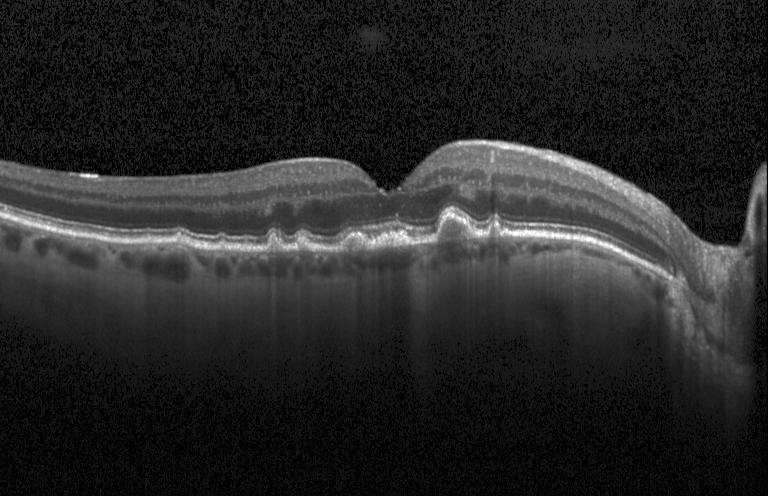

Multiple drusen.